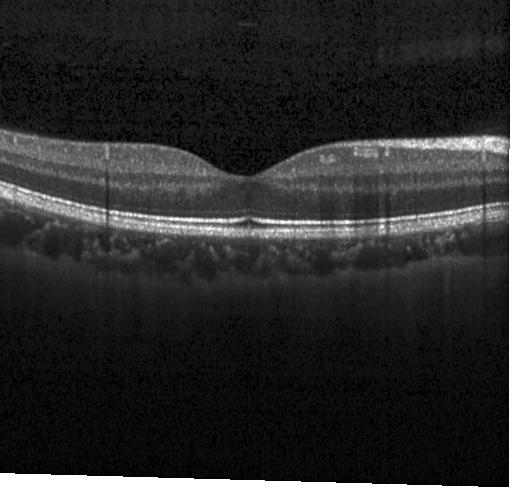

Through the macula · Heidelberg Spectralis · spectral-domain OCT · OCT line scan
The scan shows no CNV, no DME, and no drusen.